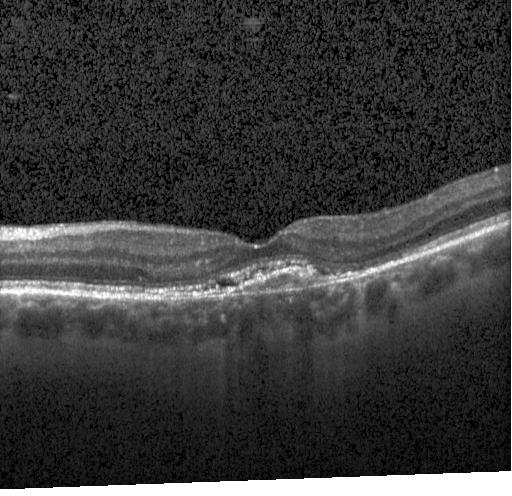

Heidelberg Spectralis OCT system, horizontal scan through the fovea, OCT line scan — The scan shows a choroidal neovascular membrane.